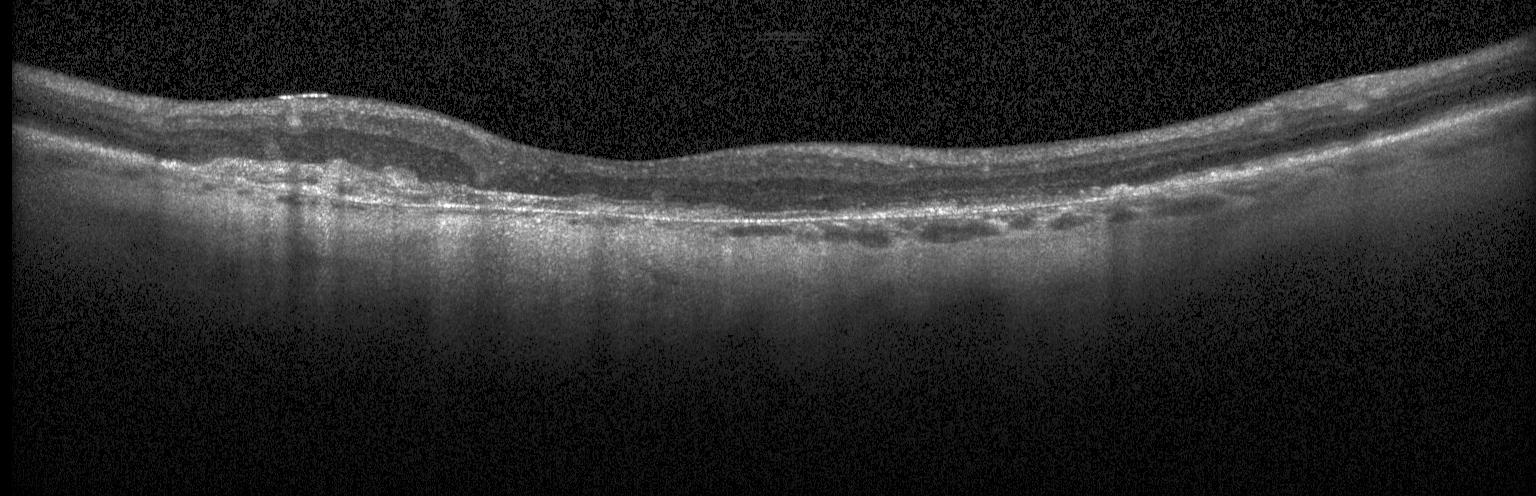 Retinal OCT B-scan, centered on the fovea. Finding: choroidal neovascularization.